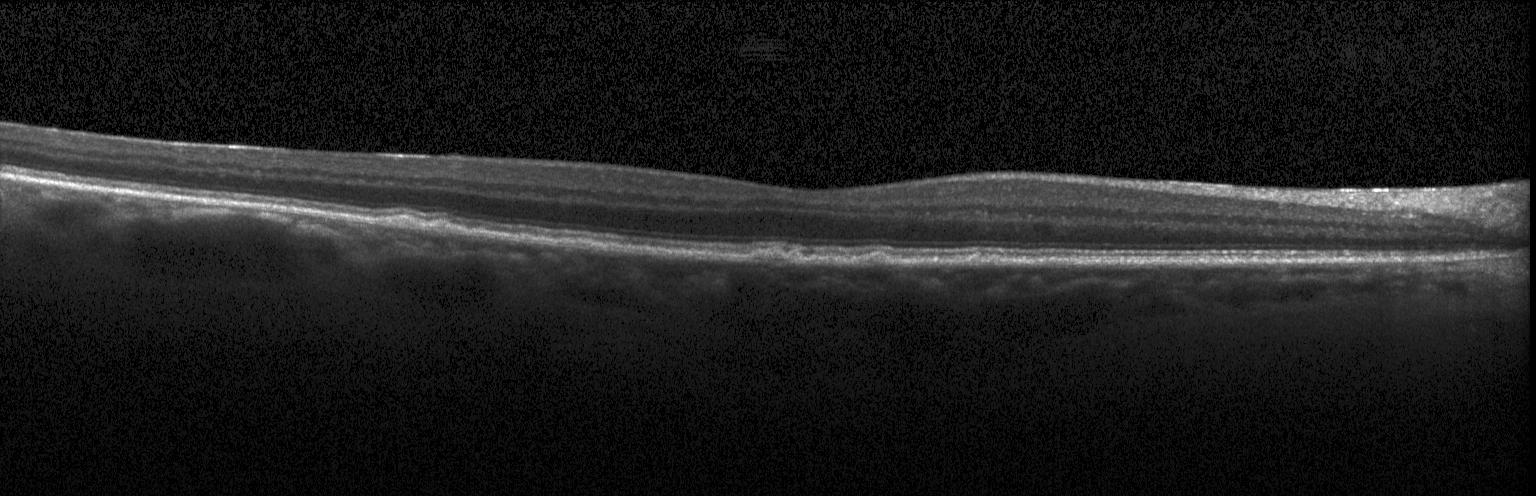

Impression: drusen.